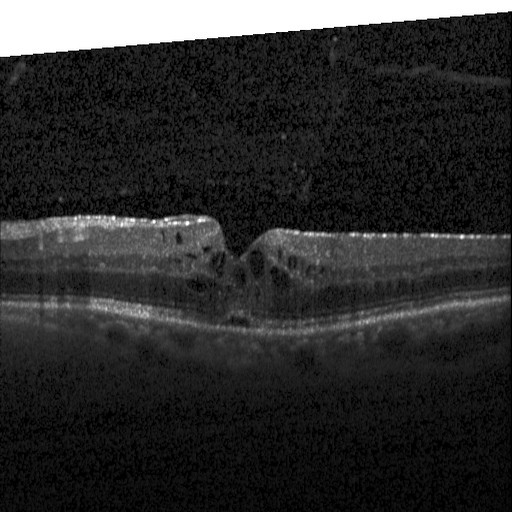

SD-OCT · centered on the fovea · optical coherence tomography scan — Diagnosis: diabetic macular edema.